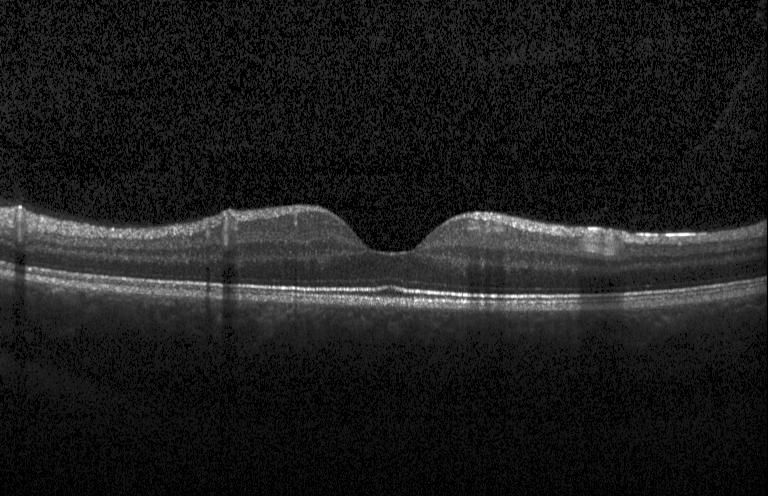
Impression: no choroidal neovascularization, diabetic macular edema, or drusen.